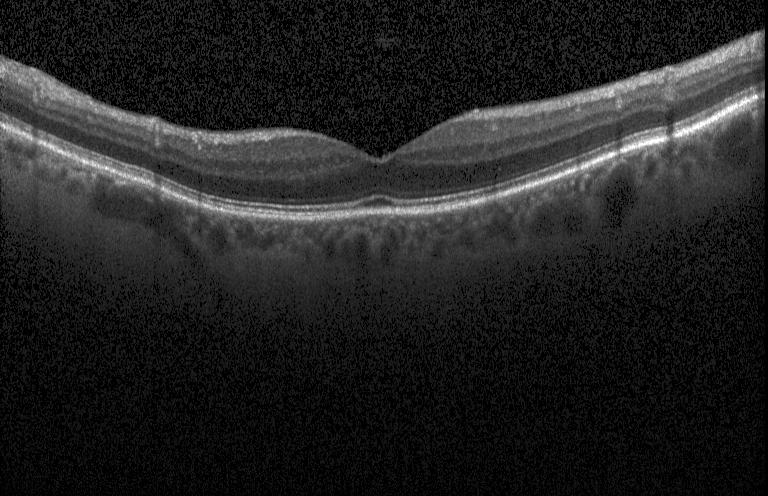
Finding: no evidence of CNV, DME, or drusen.